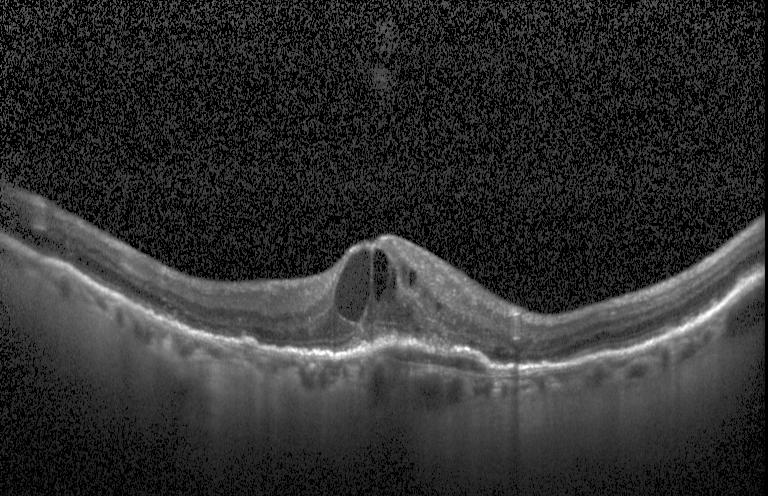 OCT line scan · spectral-domain OCT · centered on the fovea. Impression: a choroidal neovascular membrane.